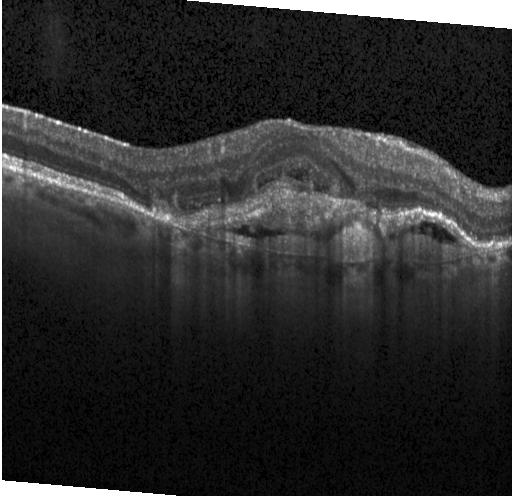

Macular OCT demonstrating a choroidal neovascular membrane.